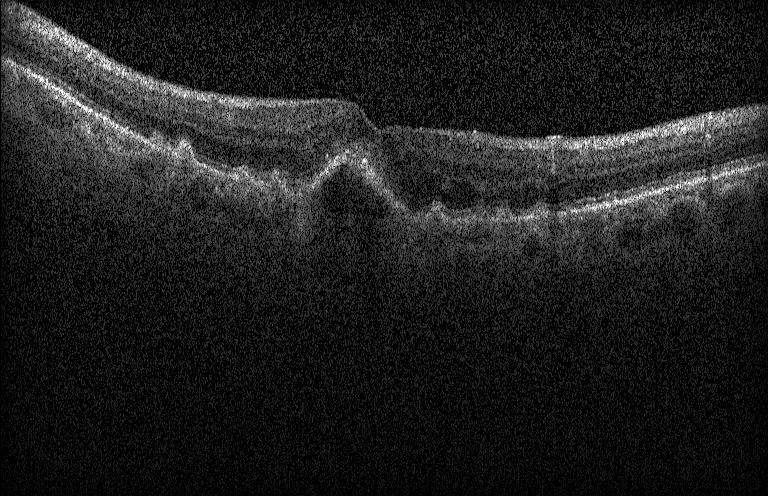
This B-scan demonstrates CNV.